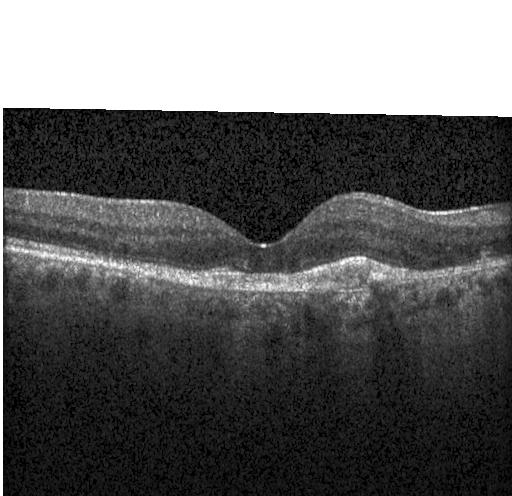 Dx: a choroidal neovascular membrane.